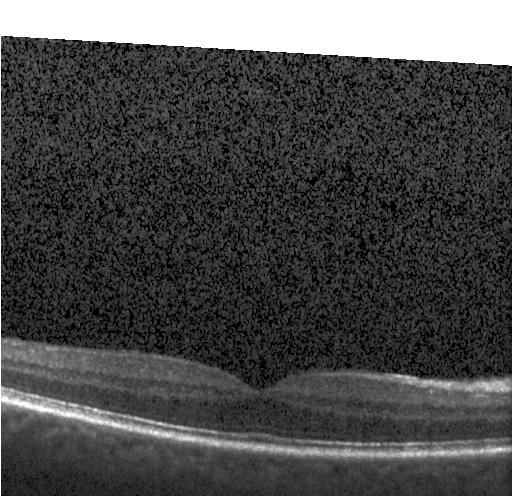

OCT B-scan · spectral-domain optical coherence tomography · acquired on a Heidelberg Spectralis · through the macula
Impression: no choroidal neovascularization, no diabetic macular edema, and no drusen.